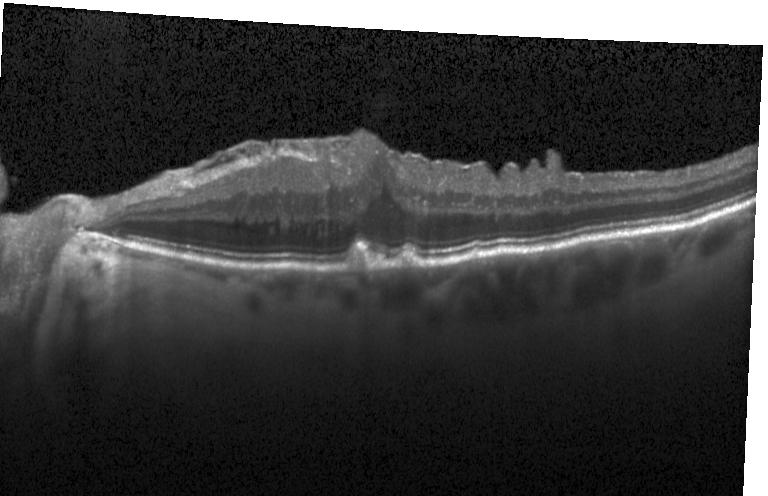
Centered on the fovea, acquired on a Heidelberg Spectralis, retinal OCT B-scan.
Impression: sub-RPE drusenoid deposits.